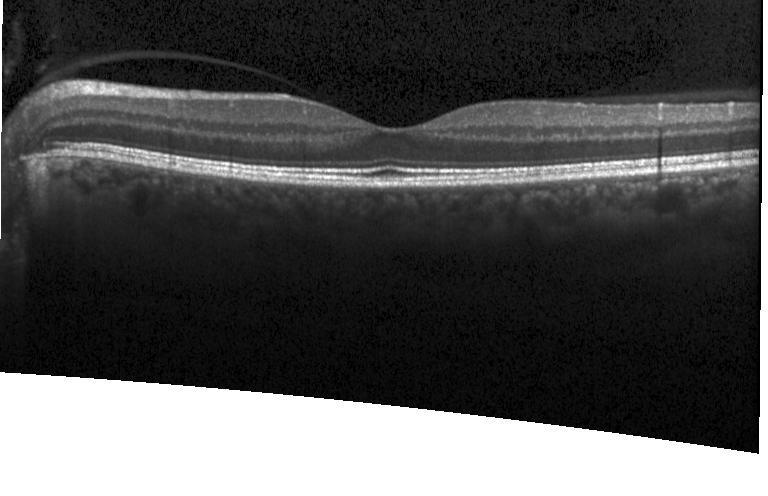 Instrument: Heidelberg Spectralis. Retinal OCT B-scan. Spectral-domain optical coherence tomography. Through the macula.
Finding: no CNV, no DME, and no drusen.